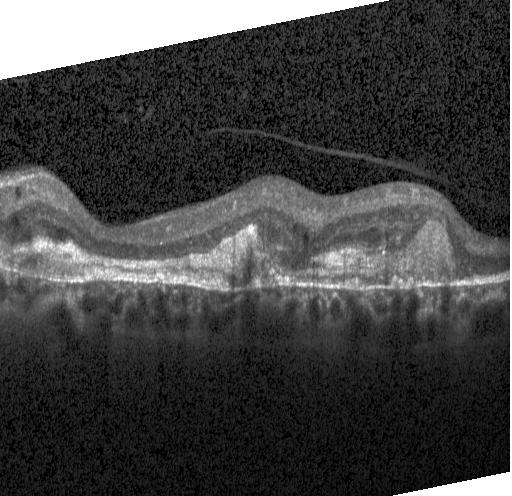 Retinal OCT cross-section · macular scan · instrument: Heidelberg Spectralis · spectral-domain optical coherence tomography.
Impression: CNV.